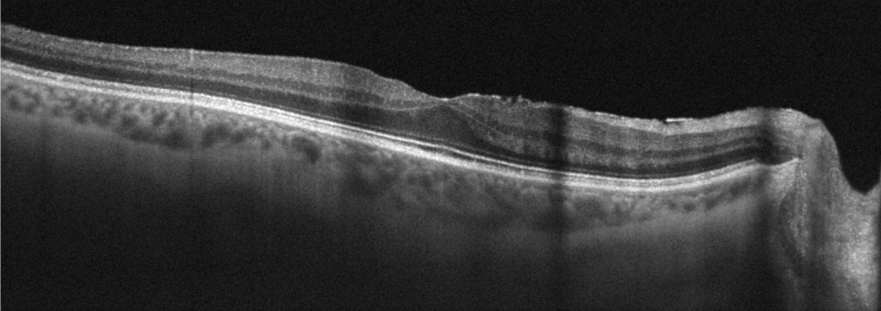
Optovue Avanti RTVue XR, retinal OCT cross-section
Impression: epiretinal membrane.